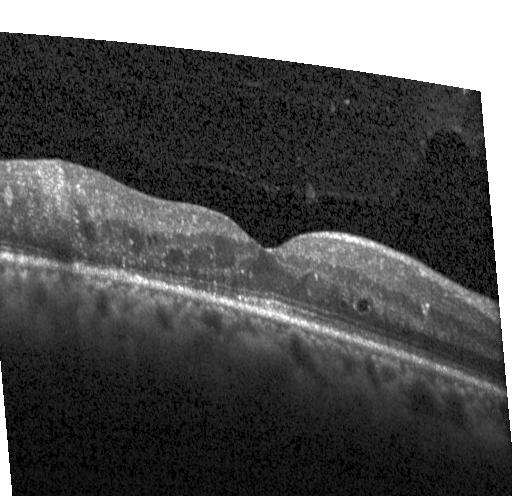
Impression: diabetic macular edema (DME).